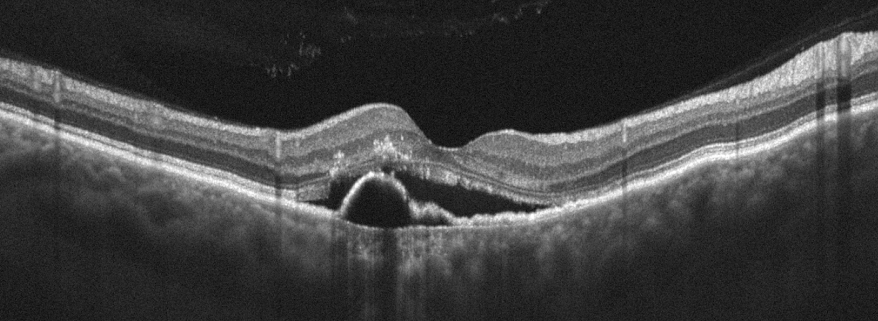 Impression: AMD.